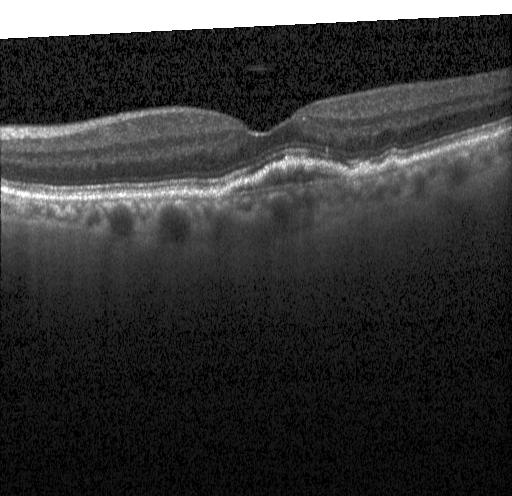 Retinal OCT B-scan, spectral-domain optical coherence tomography — Macular OCT: a choroidal neovascular membrane.